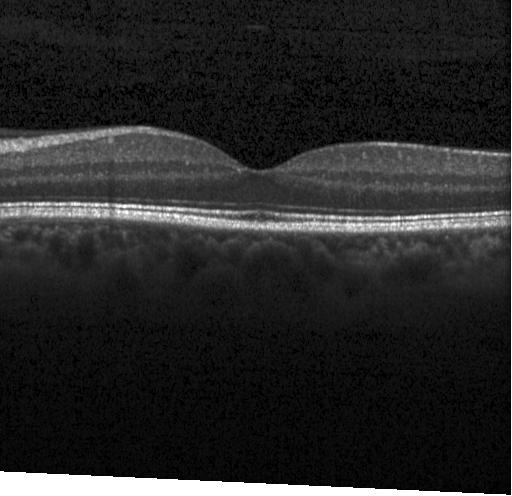
Assessment: no evidence of CNV, DME, or drusen.